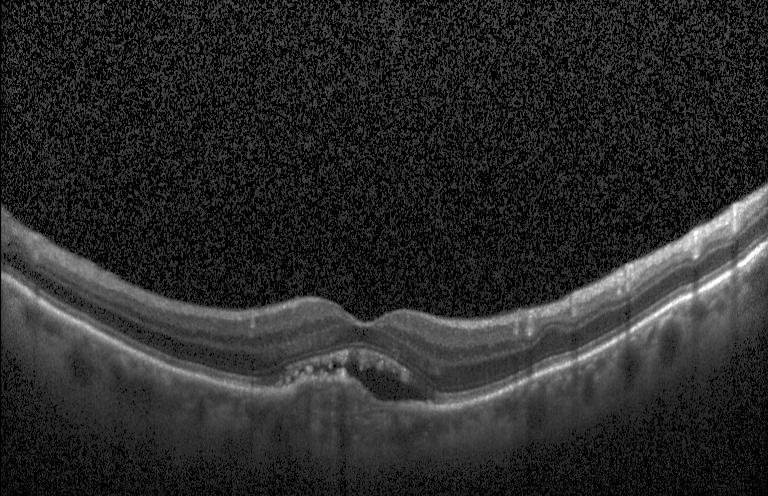
OCT B-scan · fovea-centered — This B-scan demonstrates a choroidal neovascular membrane.